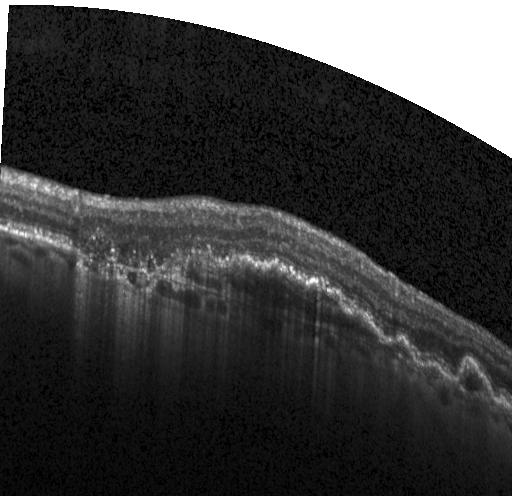

Instrument: Heidelberg Spectralis; SD-OCT; retinal OCT B-scan — Diagnosis: a choroidal neovascular membrane.